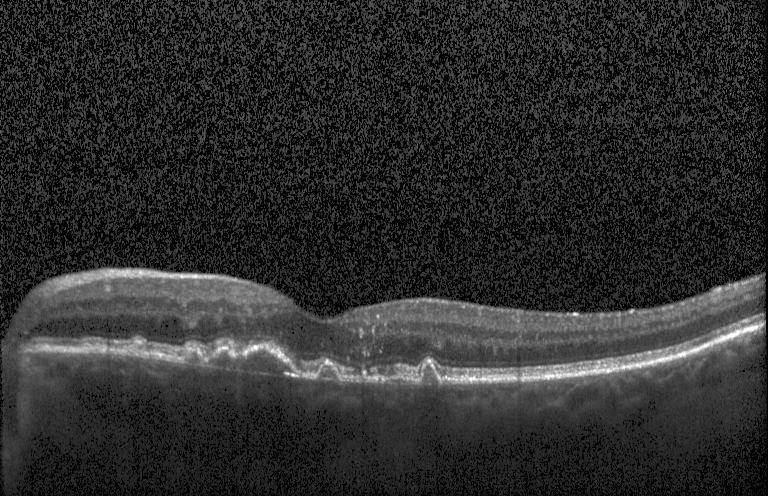
OCT B-scan.
Impression: a choroidal neovascular membrane.